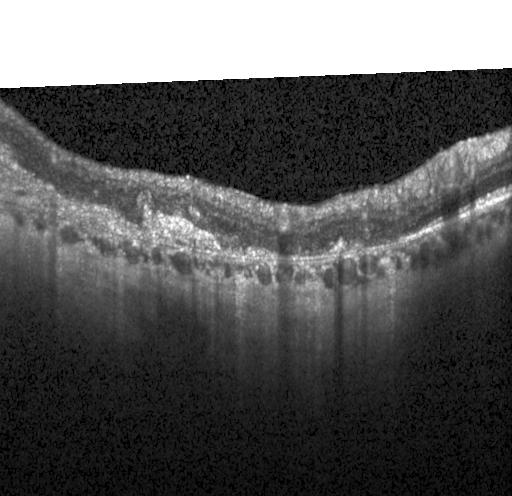

SD-OCT · optical coherence tomography B-scan · fovea-centered
Finding: a choroidal neovascular membrane.